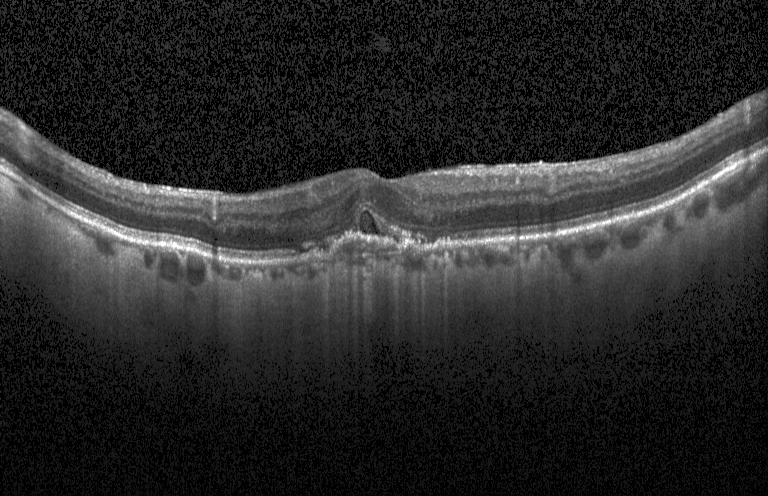
Impression: a choroidal neovascular membrane.